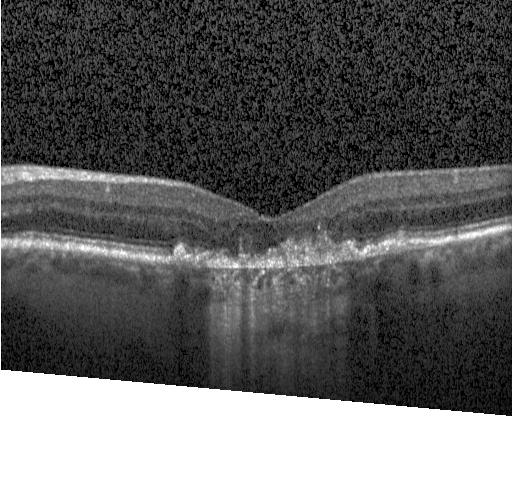
Acquired on a Heidelberg Spectralis, OCT B-scan.
Assessment: choroidal neovascularization.